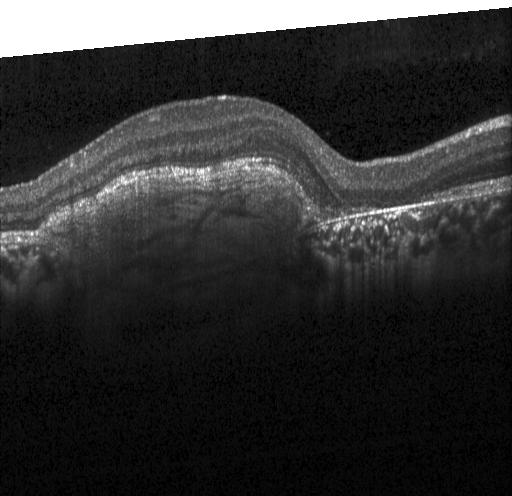

This B-scan demonstrates CNV.